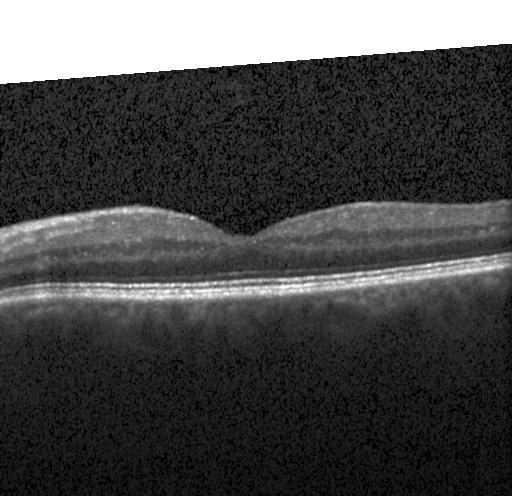

Centered on the fovea. OCT line scan. No evidence of choroidal neovascularization, diabetic macular edema, or drusen.